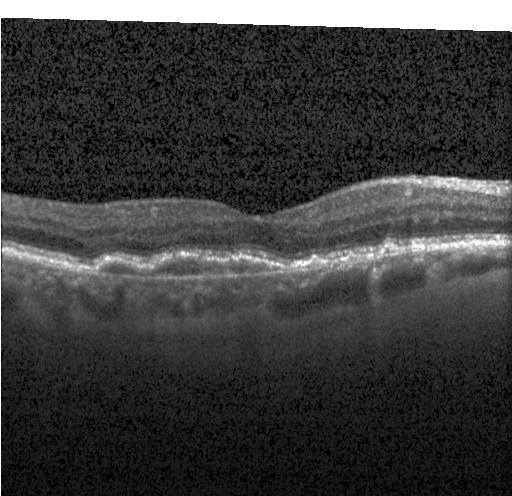

Optical coherence tomography B-scan. Dx: a choroidal neovascular membrane.